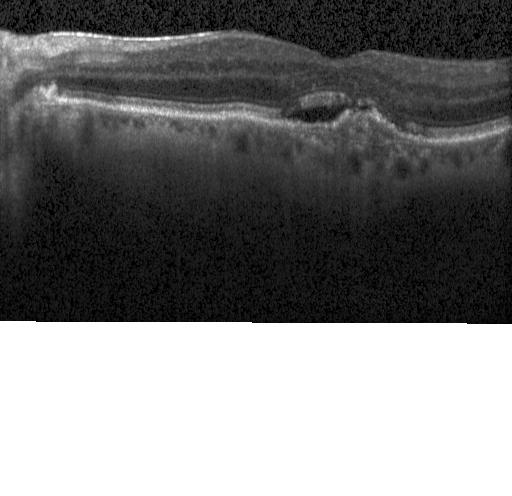 OCT line scan — Assessment: choroidal neovascularization.